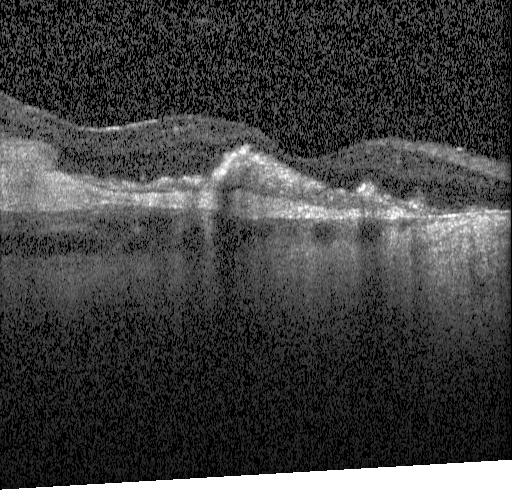
OCT B-scan, spectral-domain OCT
A choroidal neovascular membrane.